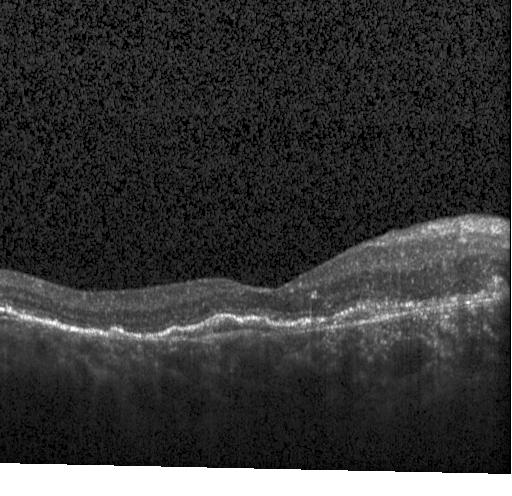

OCT B-scan showing a choroidal neovascular membrane.